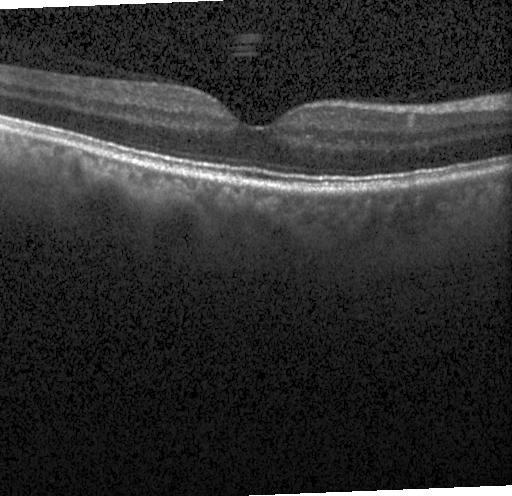 Impression: neither choroidal neovascularization, diabetic macular edema, nor drusen.